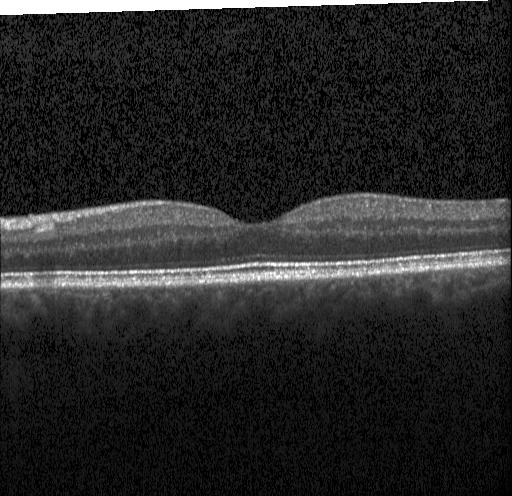

This B-scan demonstrates no CNV, DME, or drusen.